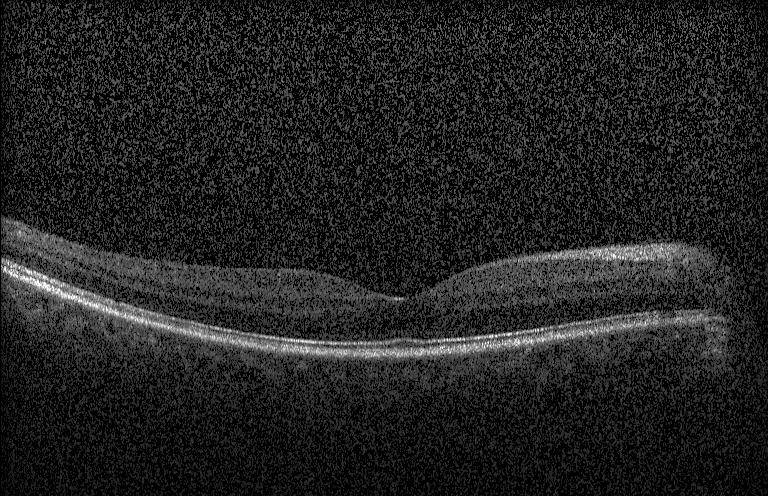

Heidelberg Spectralis; optical coherence tomography scan; spectral-domain optical coherence tomography
Dx: no evidence of choroidal neovascularization, diabetic macular edema, or drusen.